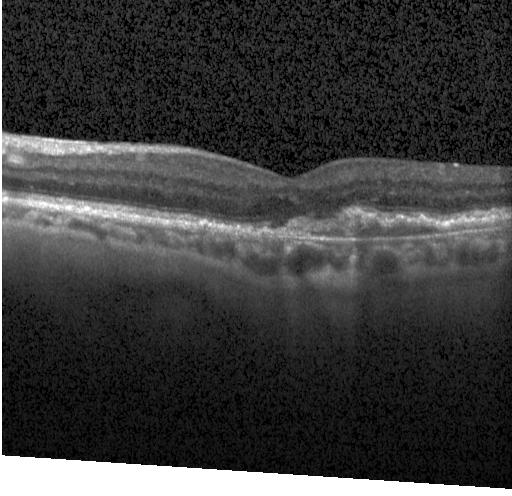

Acquired on a Heidelberg Spectralis. Macular scan. Spectral-domain OCT. Optical coherence tomography B-scan — Macular OCT: a choroidal neovascular membrane.